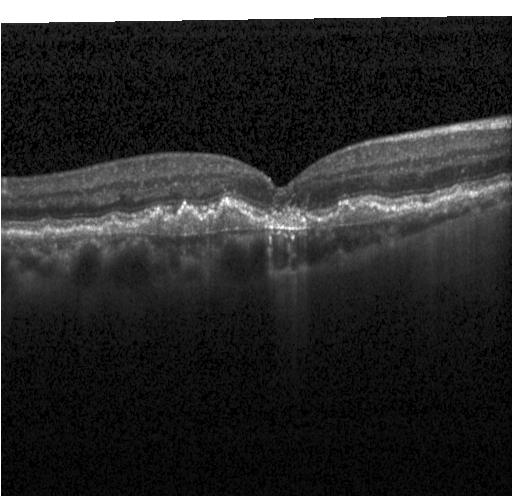 Retinal OCT cross-section. Diagnosis: a choroidal neovascular membrane.